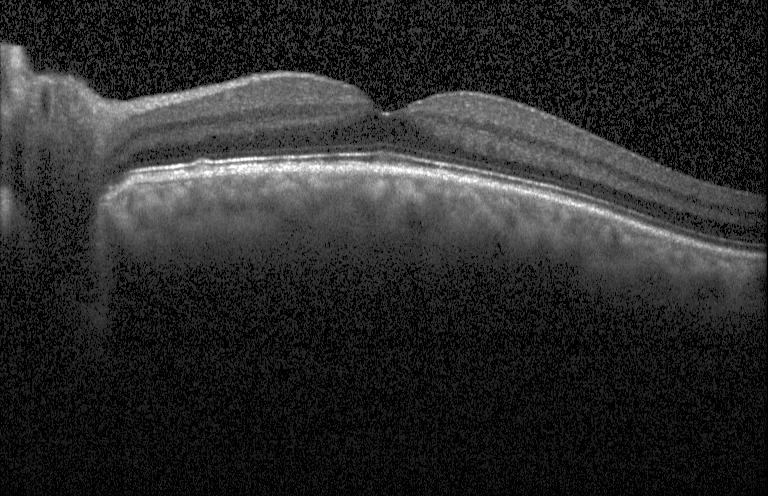

Impression: no choroidal neovascularization, diabetic macular edema, or drusen.